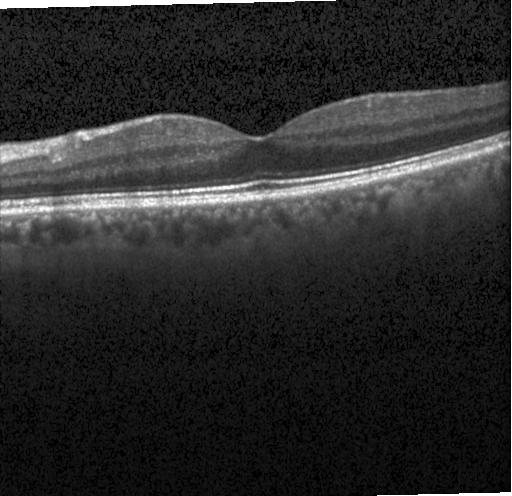 Retinal OCT B-scan · SD-OCT. Impression: no evidence of choroidal neovascularization, diabetic macular edema, or drusen.